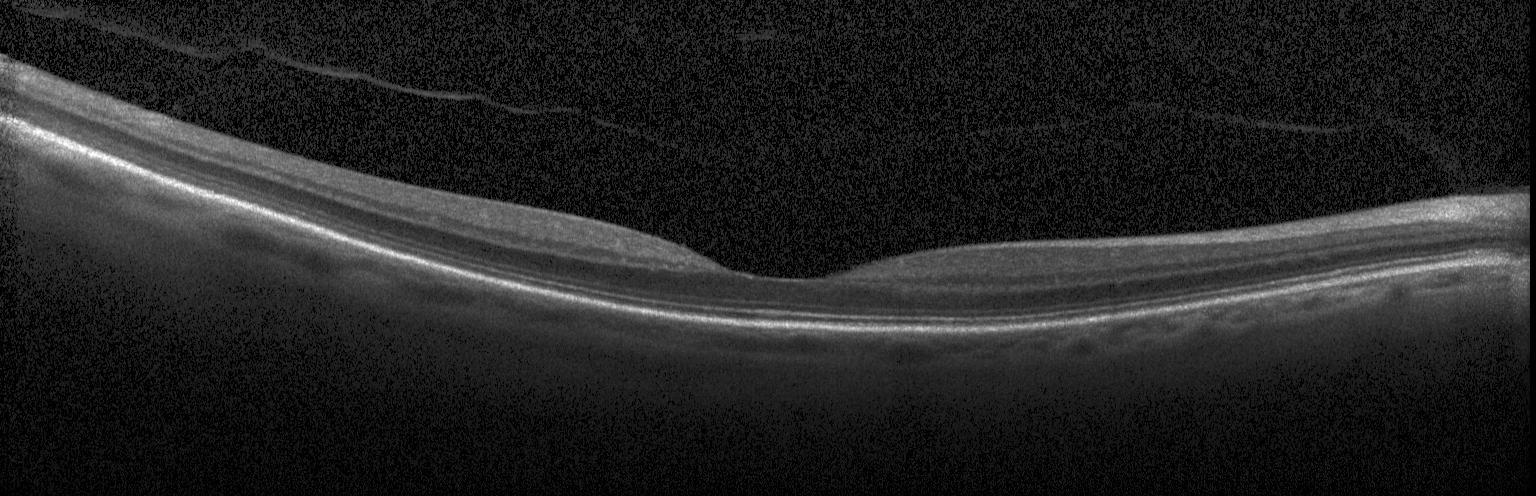

OCT B-scan · Heidelberg Spectralis OCT system
Finding: no CNV, no DME, and no drusen.